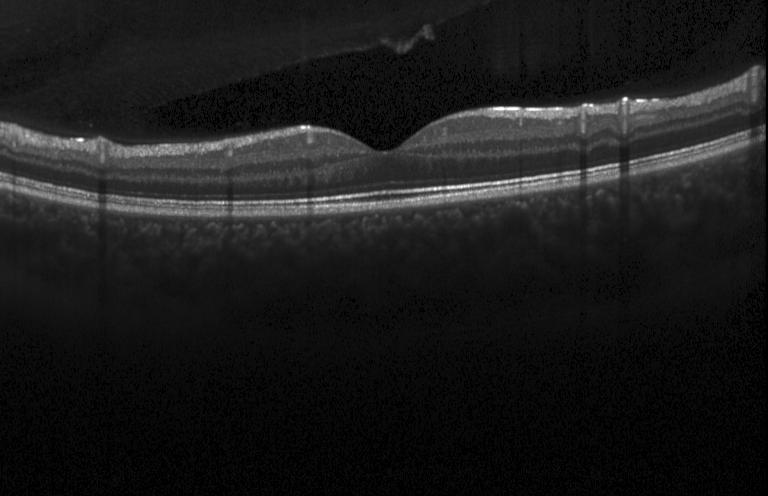

Impression: no evidence of choroidal neovascularization, diabetic macular edema, or drusen.